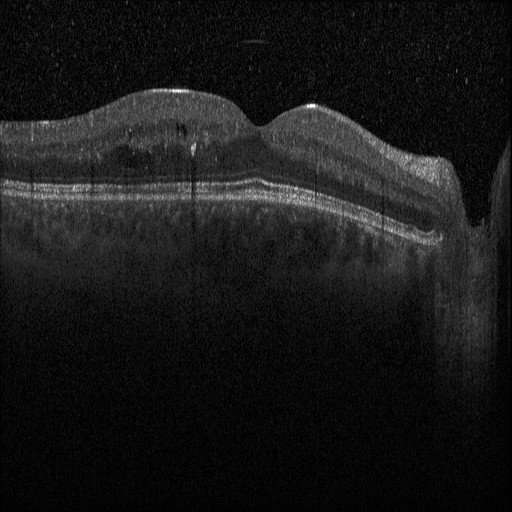
OCT line scan, acquired on a Heidelberg Spectralis, SD-OCT, centered on the fovea. OCT finding: diabetic macular edema (DME).